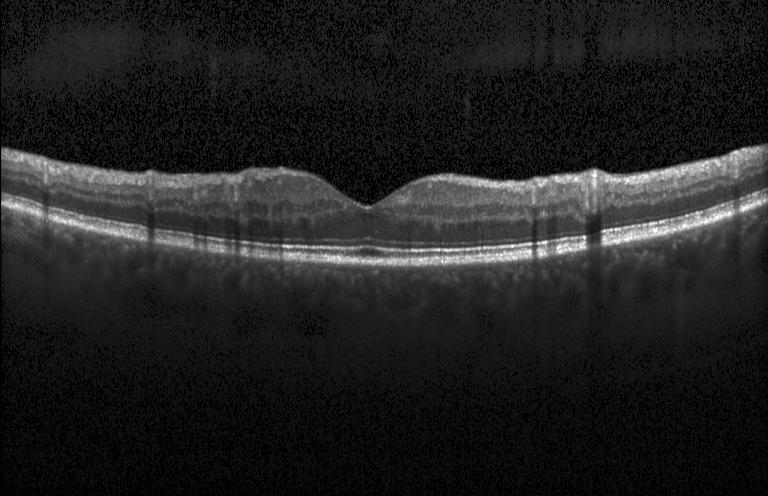
Optical coherence tomography B-scan
The scan shows no choroidal neovascularization, diabetic macular edema, or drusen.